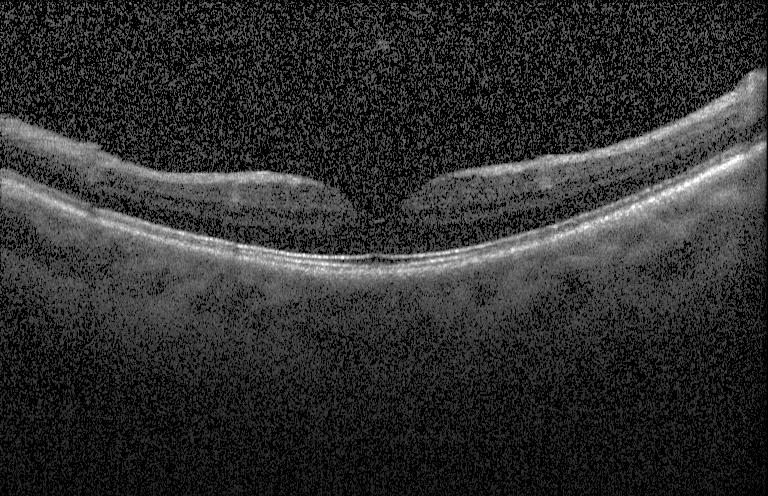

Spectral-domain optical coherence tomography; Heidelberg Spectralis; macular scan; retinal OCT cross-section
Impression: no choroidal neovascularization, diabetic macular edema, or drusen.